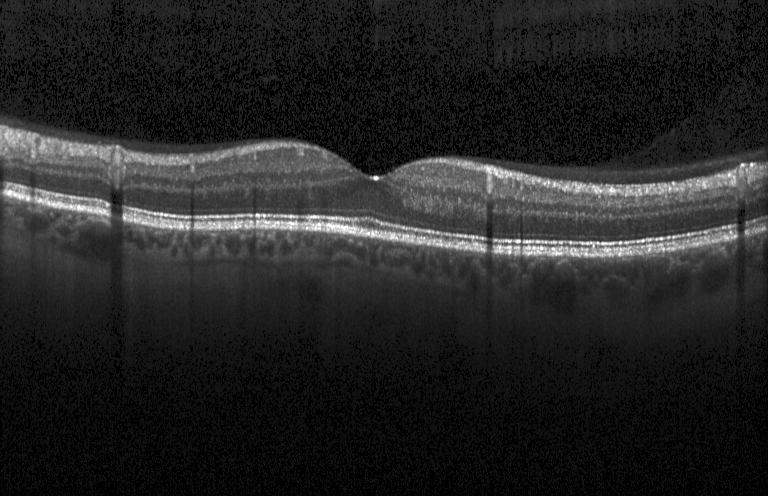 OCT line scan — Finding: no choroidal neovascularization, no diabetic macular edema, and no drusen.